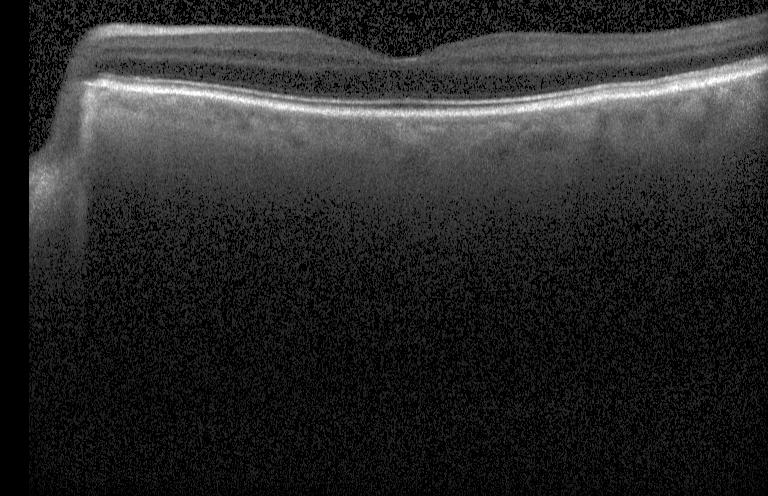

Spectral-domain OCT B-scan: no CNV, no DME, and no drusen.